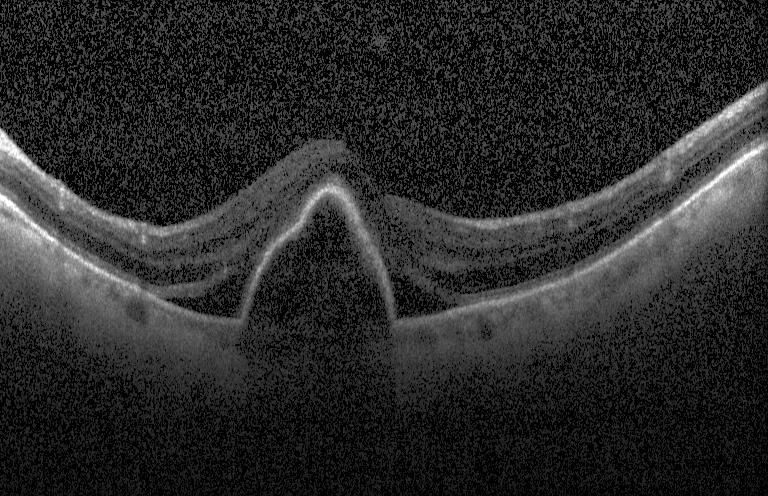

Macular scan. Optical coherence tomography scan — The scan shows a choroidal neovascular membrane.